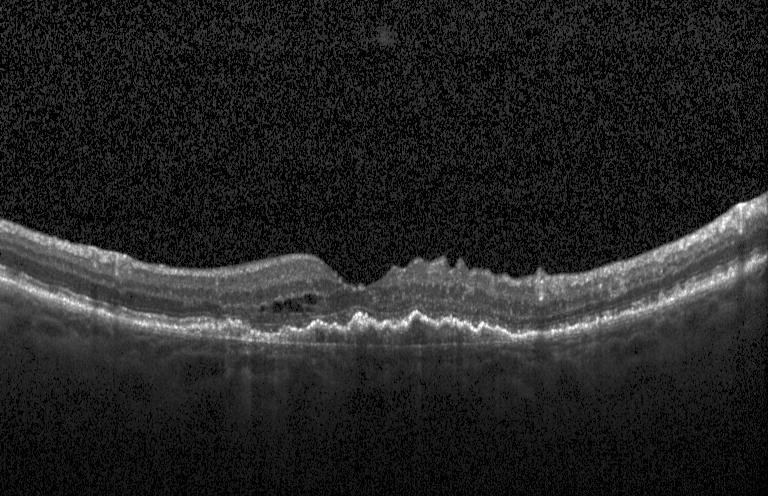 Fovea-centered, optical coherence tomography scan, SD-OCT, Heidelberg Spectralis OCT system — This B-scan demonstrates a choroidal neovascular membrane.